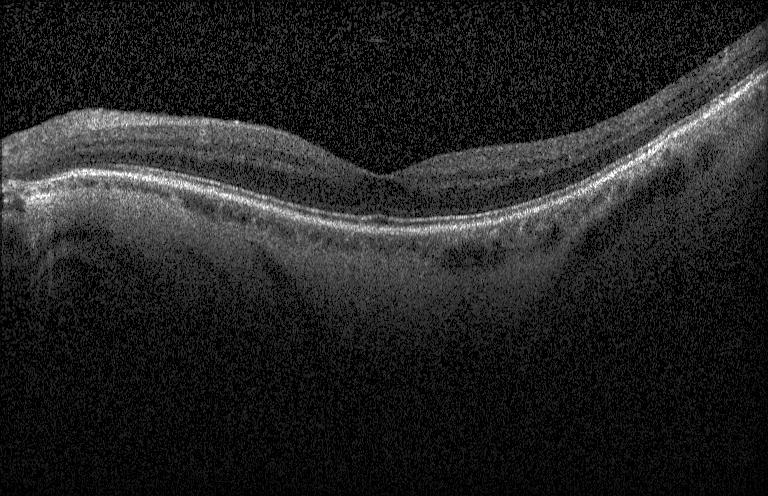
No evidence of choroidal neovascularization, diabetic macular edema, or drusen.